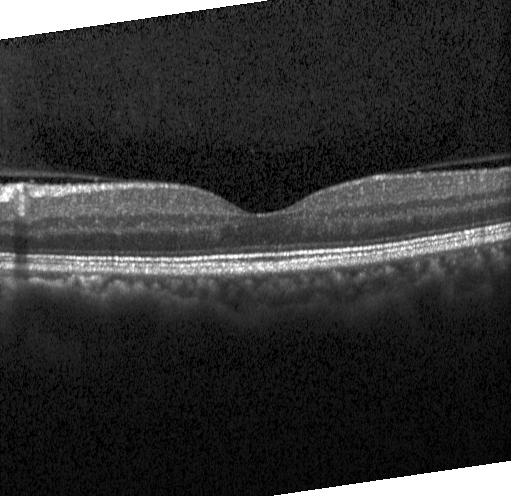

Instrument: Heidelberg Spectralis. Retinal OCT B-scan. Neither CNV, DME, nor drusen.